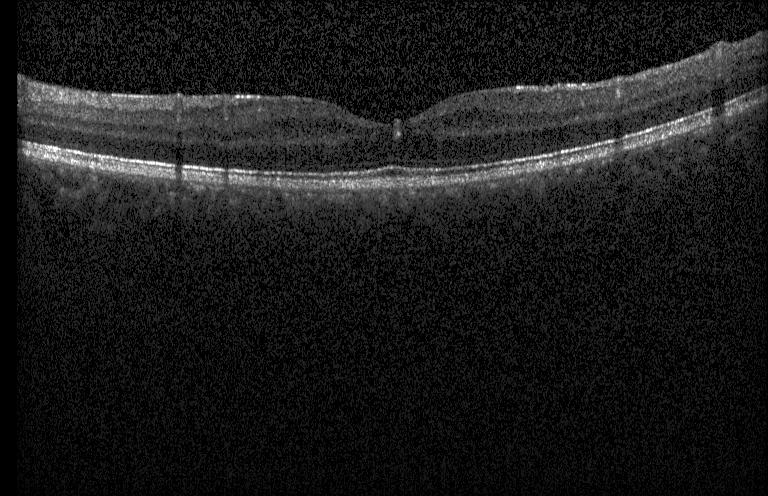

Optical coherence tomography B-scan · Heidelberg Spectralis · SD-OCT. Macular OCT: diabetic macular edema (DME).